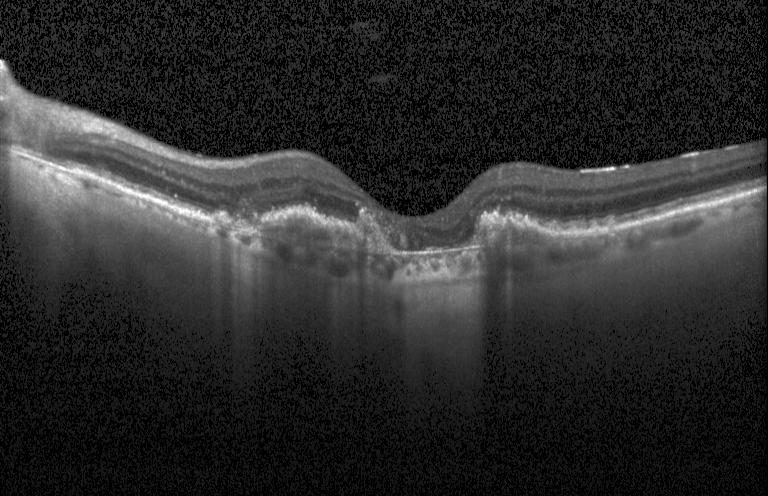 Diagnosis: CNV.